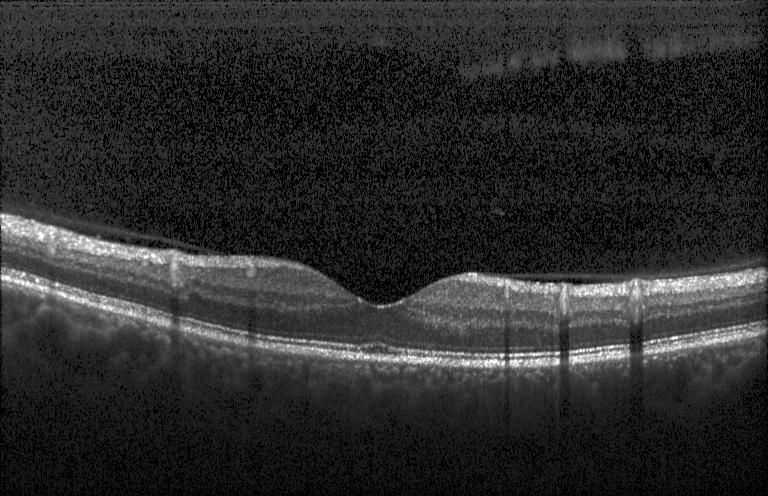

Optical coherence tomography B-scan, acquired on a Heidelberg Spectralis.
The scan shows no evidence of CNV, DME, or drusen.